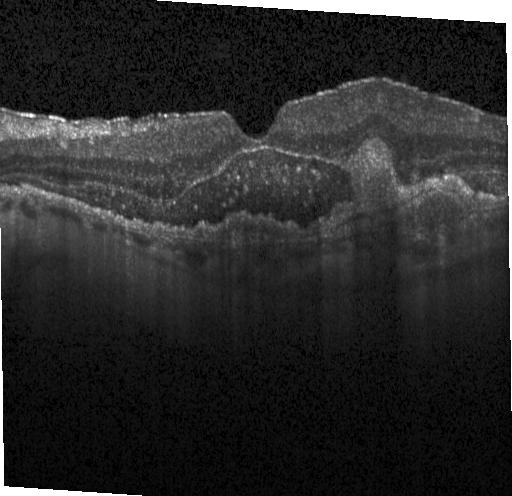

SD-OCT, retinal OCT cross-section, Heidelberg Spectralis OCT system, centered on the fovea.
OCT finding: CNV.